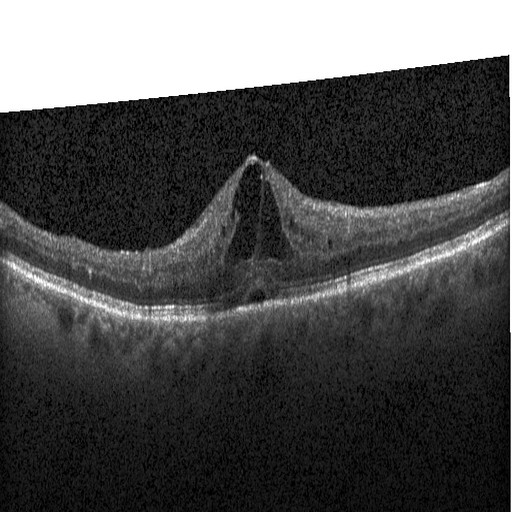

Spectral-domain OCT, retinal OCT B-scan, Heidelberg Spectralis OCT system, macular scan.
Finding: DME.